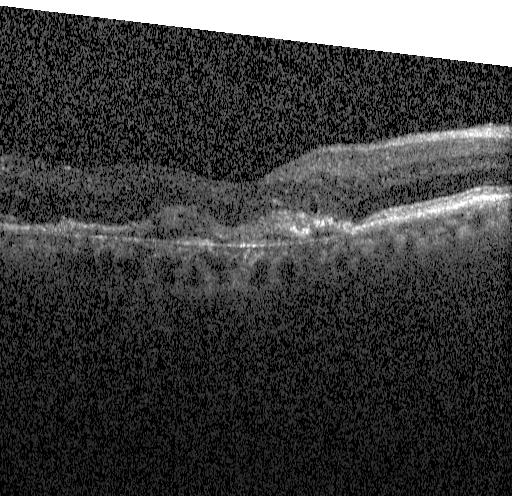
OCT line scan; centered on the fovea; acquired on a Heidelberg Spectralis; spectral-domain OCT.
Finding: choroidal neovascularization (CNV).